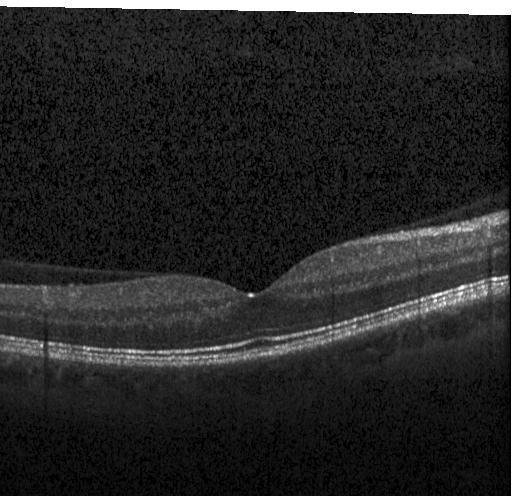

OCT B-scan · spectral-domain OCT · through the macula
The scan shows no evidence of choroidal neovascularization, diabetic macular edema, or drusen.